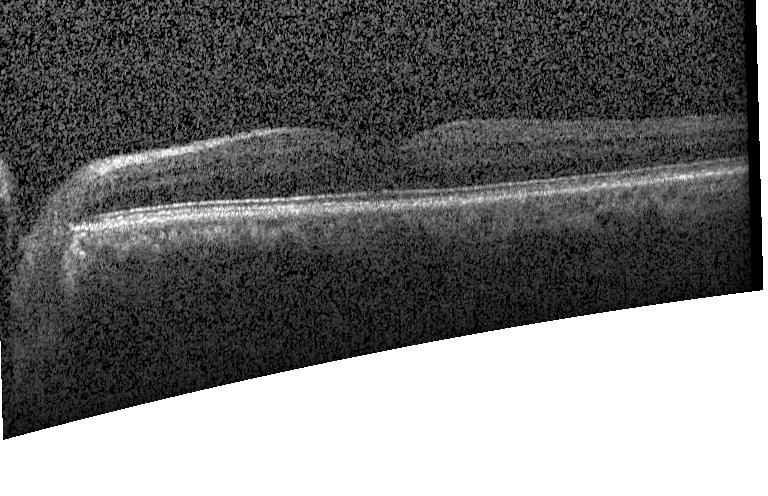
Acquired on a Heidelberg Spectralis; through the macula; optical coherence tomography scan. Assessment: neither choroidal neovascularization, diabetic macular edema, nor drusen.